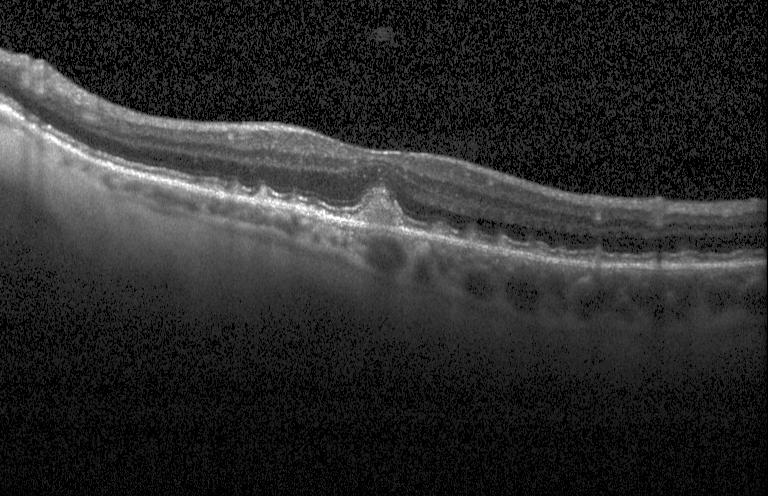
Retinal OCT B-scan
OCT finding: CNV.